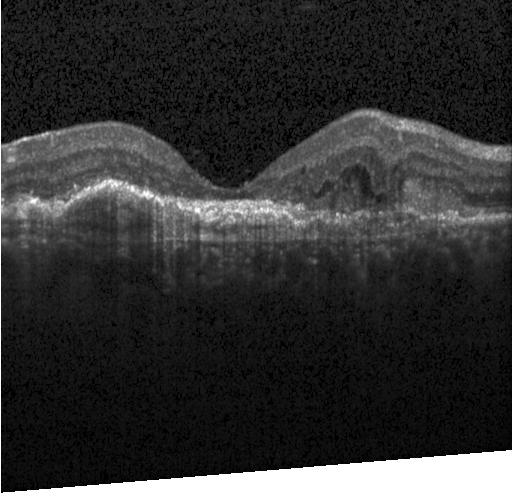

Optical coherence tomography scan.
This B-scan demonstrates a choroidal neovascular membrane.